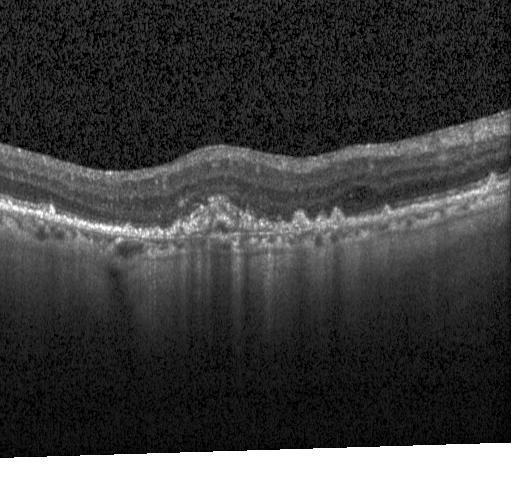
OCT finding: a choroidal neovascular membrane.